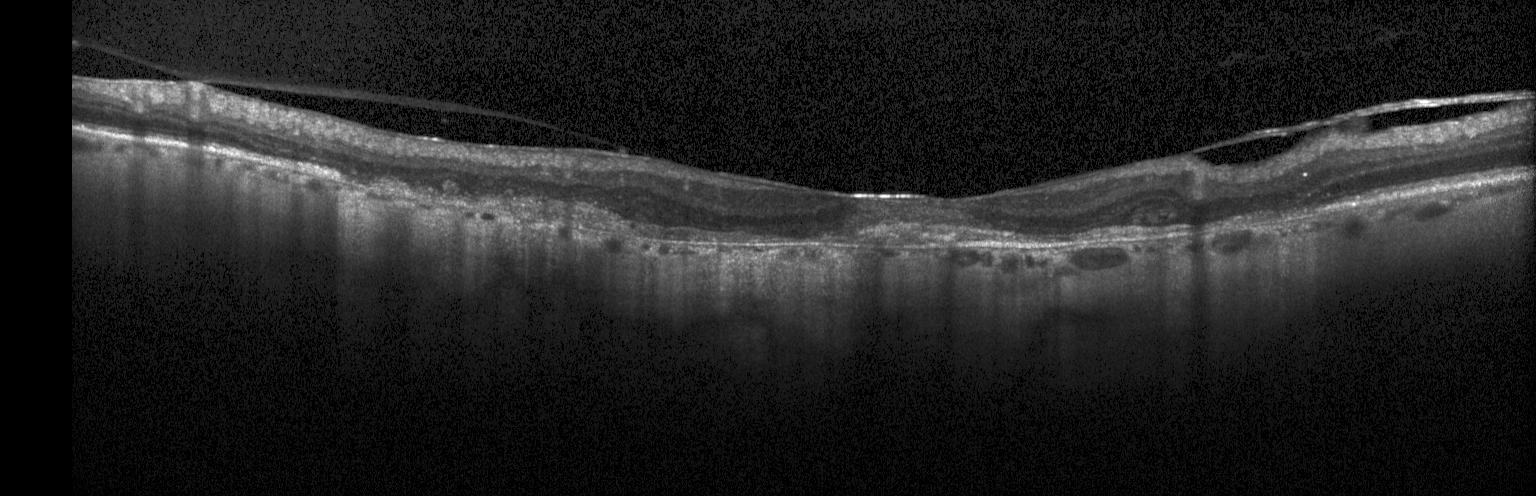
Retinal OCT B-scan, horizontal scan through the fovea
Impression: CNV.